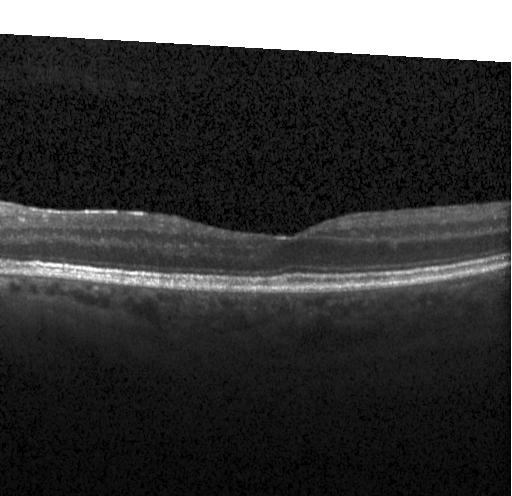
Fovea-centered, retinal OCT B-scan, spectral-domain OCT, Heidelberg Spectralis — Diagnosis: no evidence of choroidal neovascularization, diabetic macular edema, or drusen.